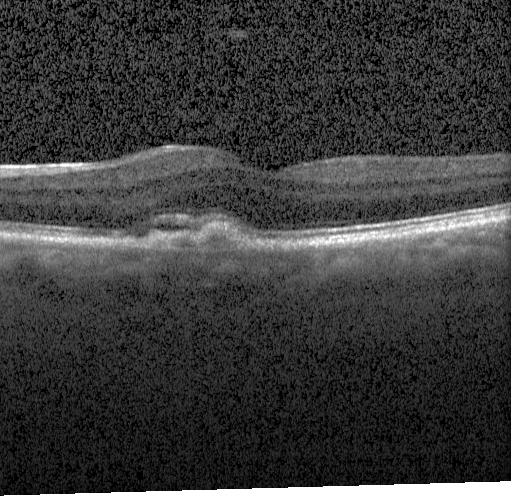
Diagnosis: a choroidal neovascular membrane.